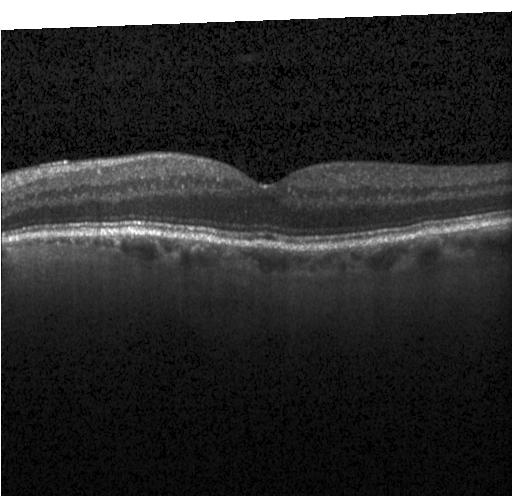

OCT finding: no choroidal neovascularization, diabetic macular edema, or drusen.